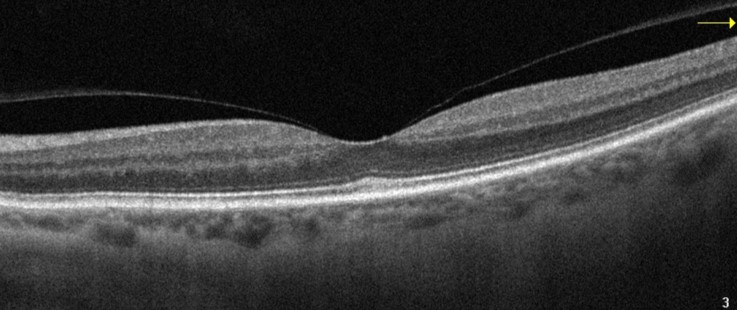 OCT line scan · macular scan. Dx: absence of AMD, DME, ERM, RAO, RVO, and vitreomacular interface disease.